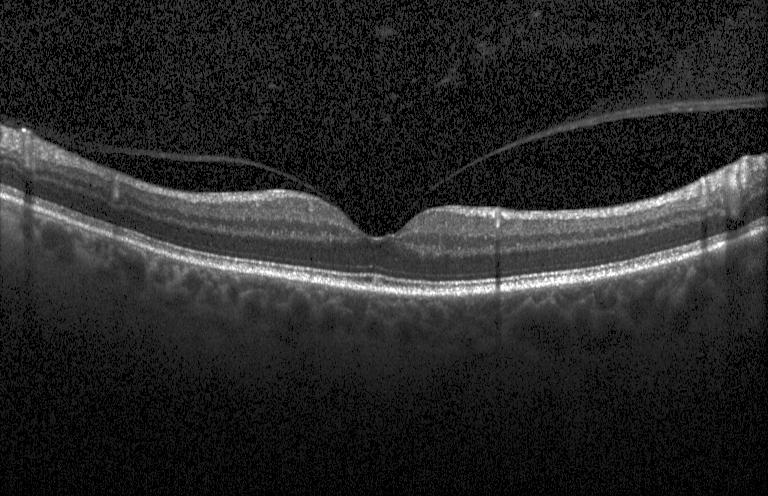

Finding: neither choroidal neovascularization, diabetic macular edema, nor drusen.